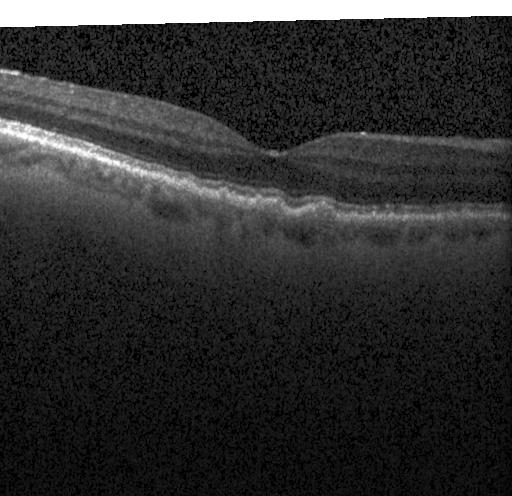 This B-scan demonstrates sub-RPE drusenoid deposits.